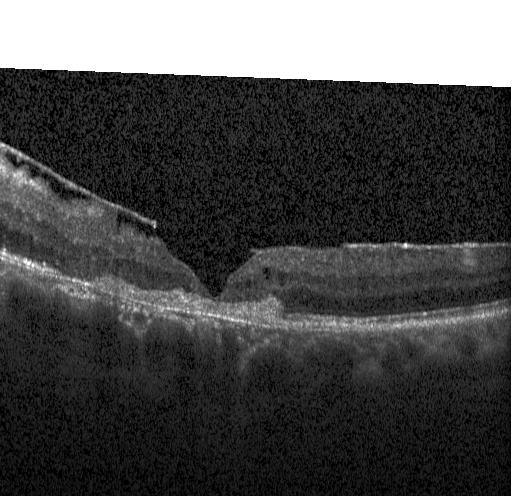 Diagnosis: a choroidal neovascular membrane.